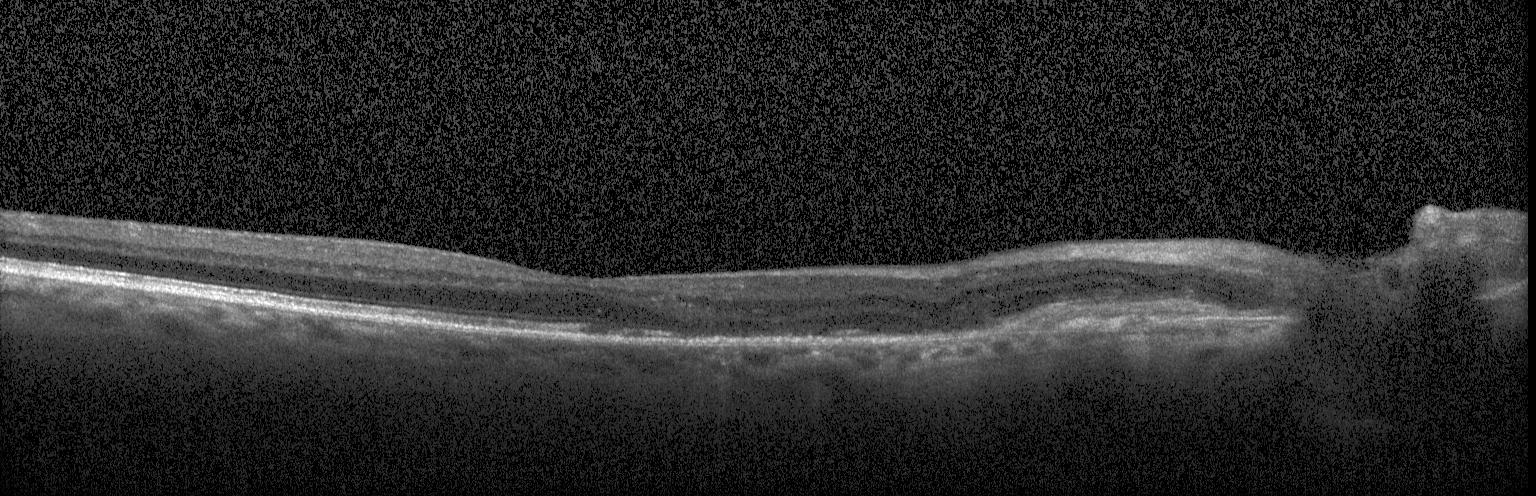
Optical coherence tomography scan
A choroidal neovascular membrane.